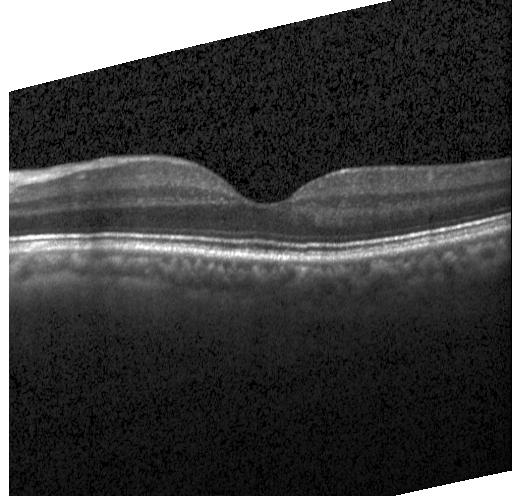
Diagnosis: no evidence of CNV, DME, or drusen.